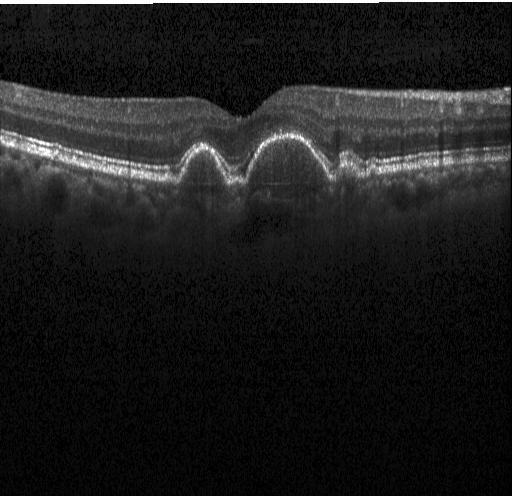

Retinal OCT cross-section showing multiple drusen.